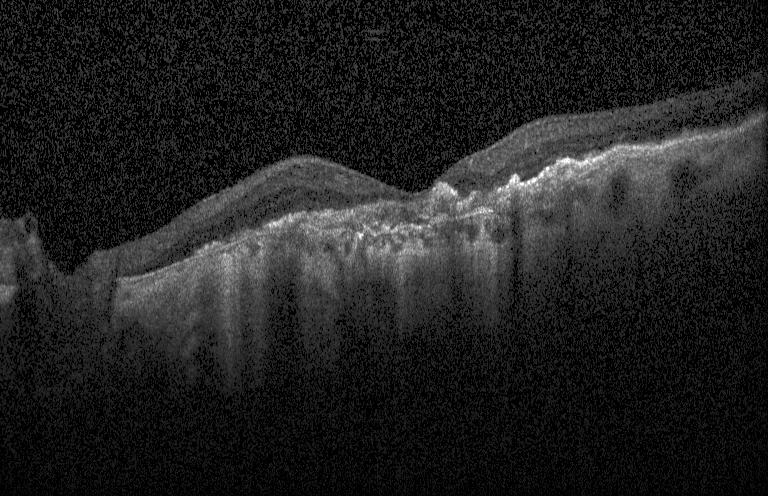

Retinal OCT cross-section
Choroidal neovascularization (CNV).